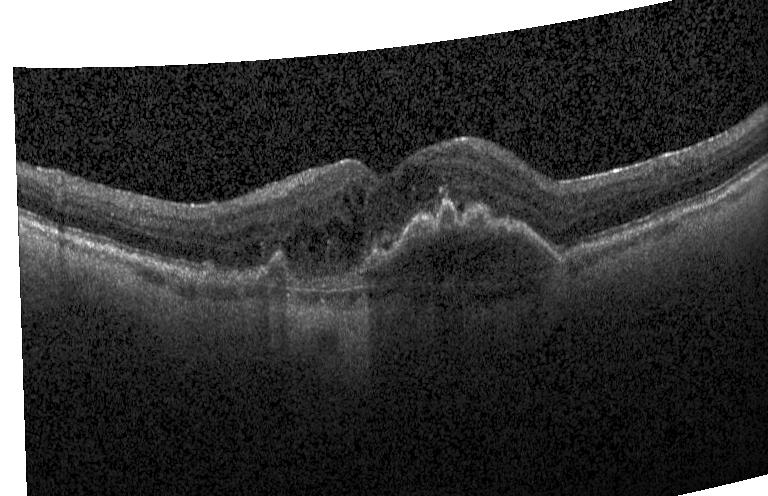
Retinal OCT cross-section; spectral-domain OCT. Diagnosis: CNV.